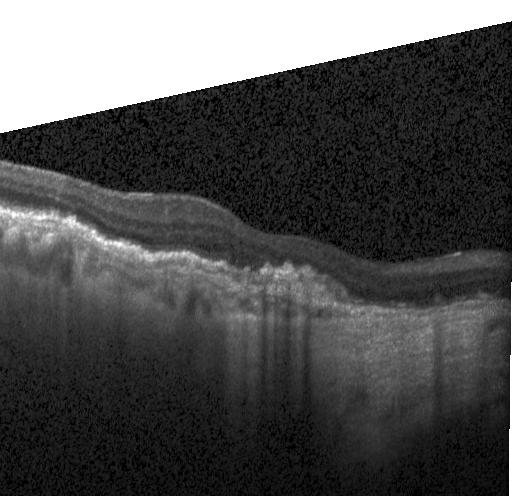

Optical coherence tomography B-scan
Impression: a choroidal neovascular membrane.